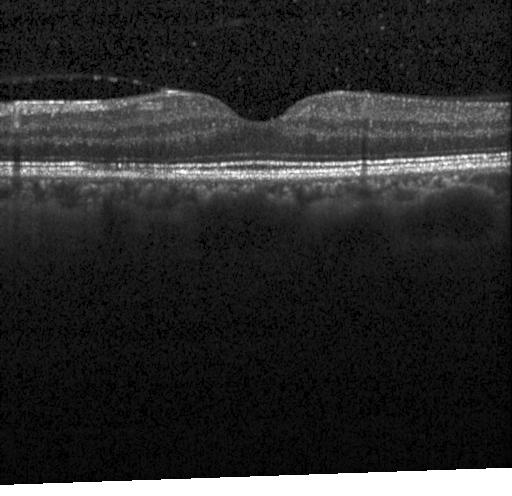
Macular OCT: no evidence of CNV, DME, or drusen.